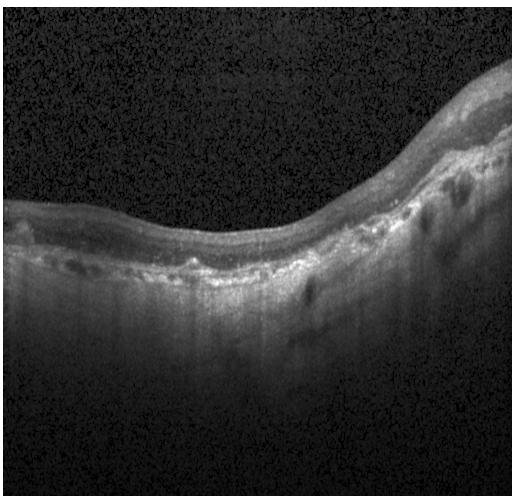 Through the macula · optical coherence tomography B-scan · SD-OCT · instrument: Heidelberg Spectralis
Impression: CNV.